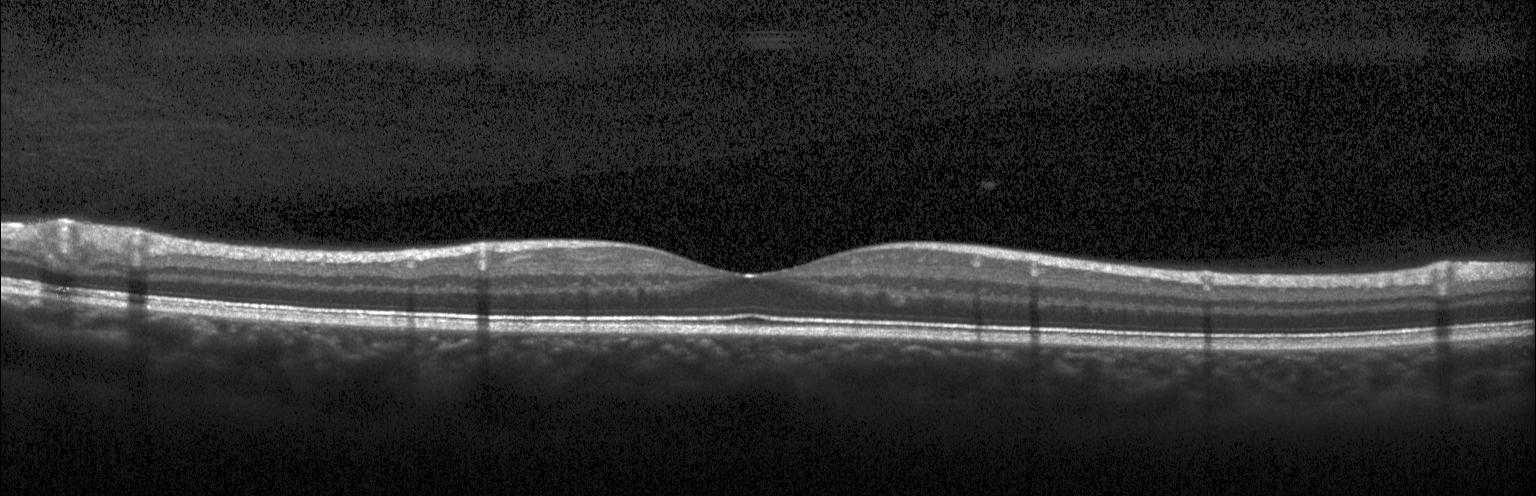

This B-scan demonstrates no choroidal neovascularization, diabetic macular edema, or drusen.